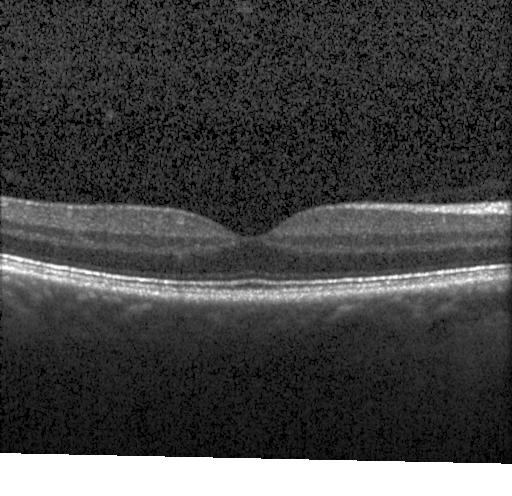
OCT B-scan — Finding: no evidence of CNV, DME, or drusen.